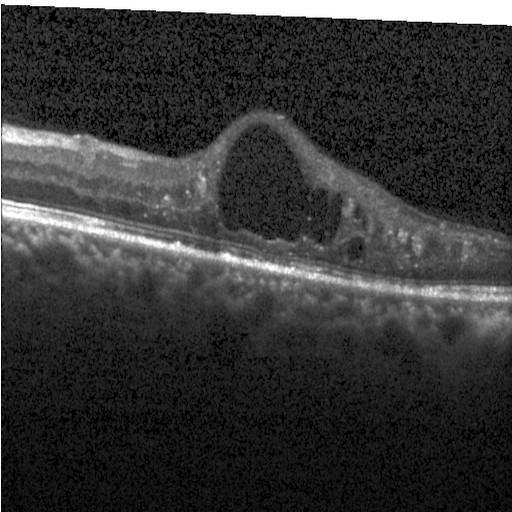 Diagnosis: diabetic macular edema.